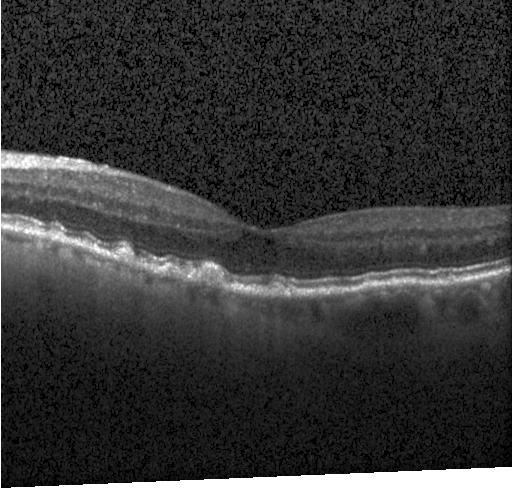 Sub-RPE drusenoid deposits.